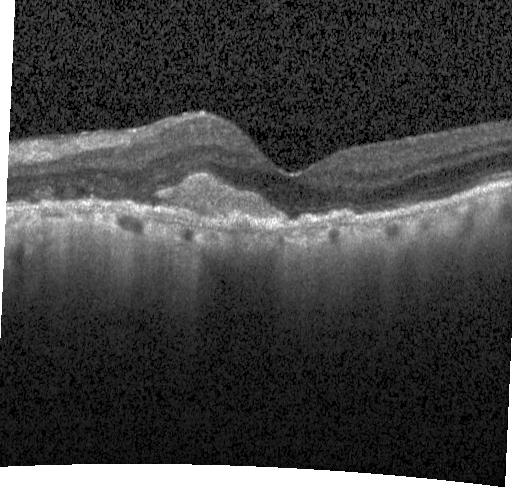
Retinal OCT B-scan.
Impression: choroidal neovascularization.